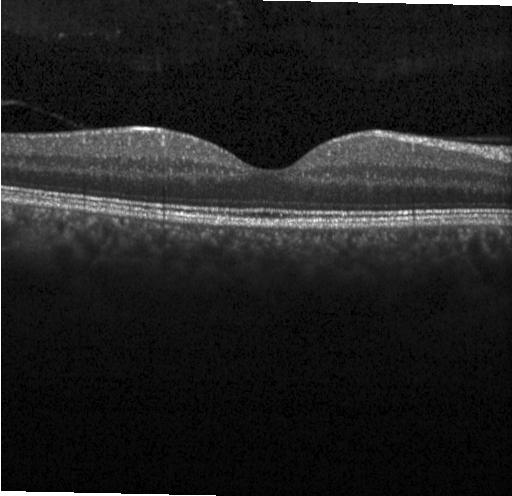 Dx: no choroidal neovascularization, diabetic macular edema, or drusen.